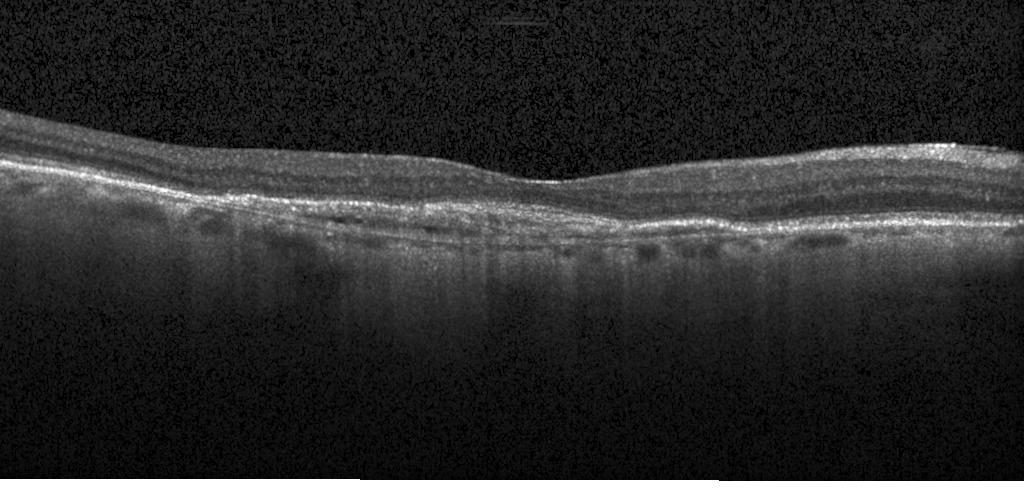

Instrument: Heidelberg Spectralis, retinal OCT cross-section.
Choroidal neovascularization (CNV).